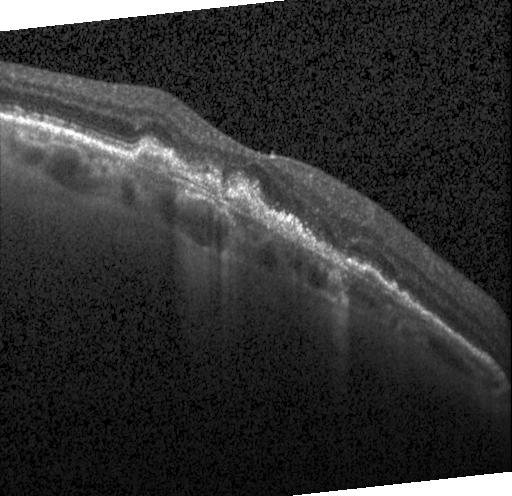 OCT B-scan showing CNV.